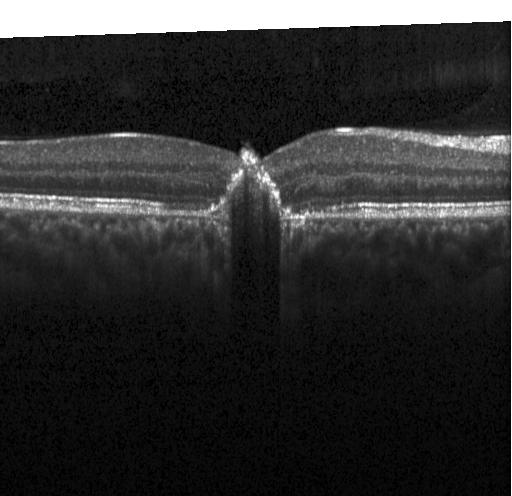

Finding: a choroidal neovascular membrane.